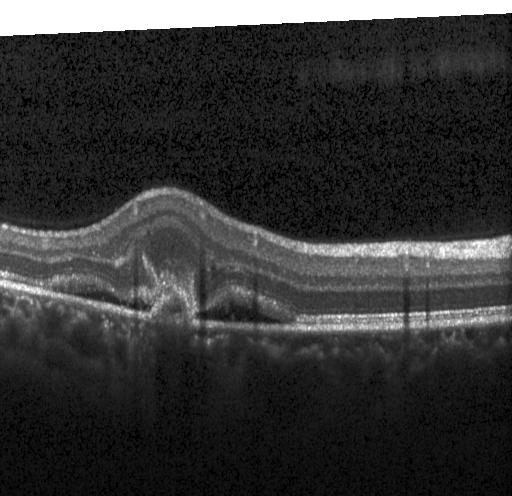 Spectral-domain OCT B-scan: CNV.